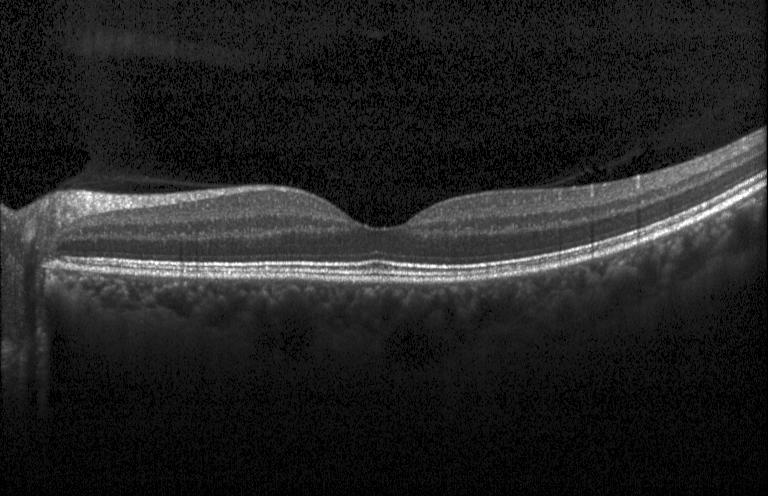
Impression: no CNV, DME, or drusen.